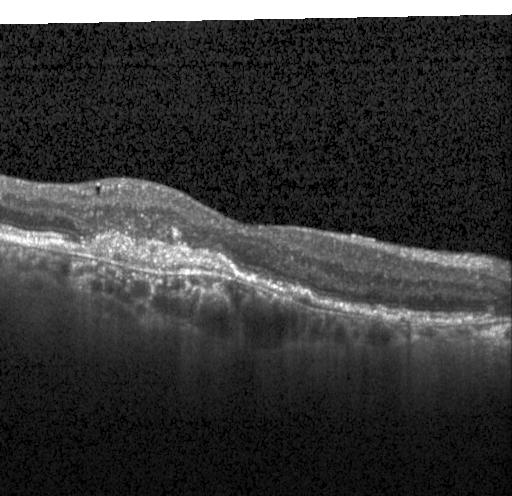
Horizontal scan through the fovea, SD-OCT, OCT B-scan — Diagnosis: a choroidal neovascular membrane.